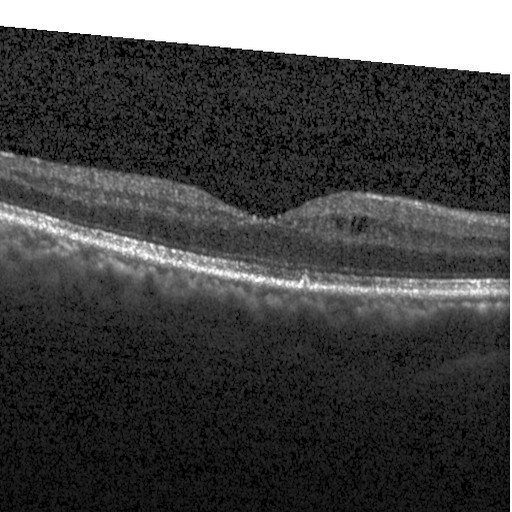
Optical coherence tomography B-scan
This B-scan demonstrates diabetic macular edema (DME).